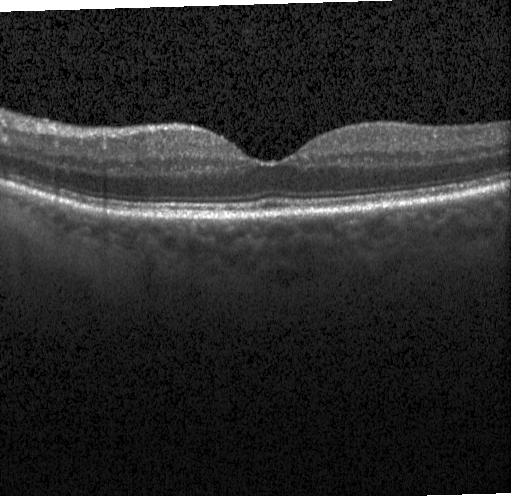

Dx: no CNV, DME, or drusen.